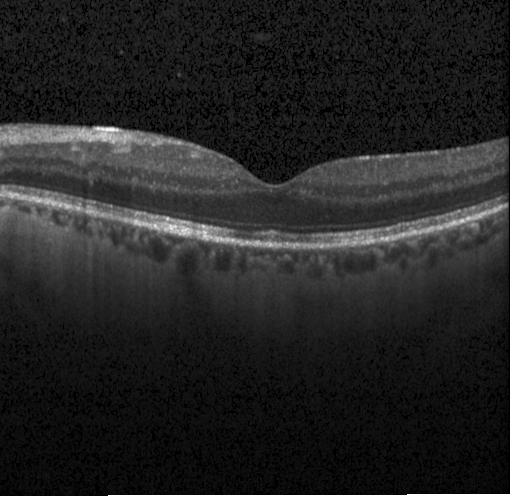 Optical coherence tomography scan — No choroidal neovascularization, diabetic macular edema, or drusen.